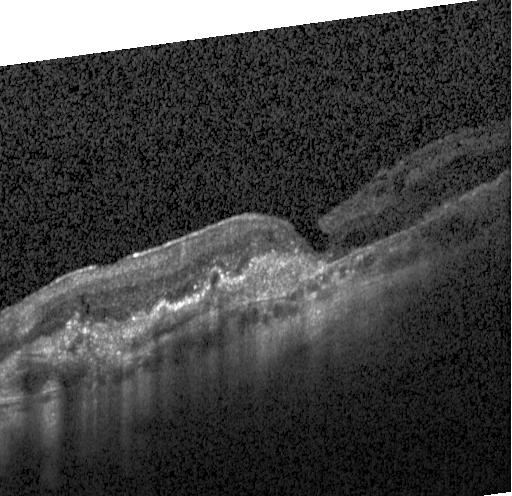 Optical coherence tomography scan · through the macula · Heidelberg Spectralis · SD-OCT — Choroidal neovascularization (CNV).